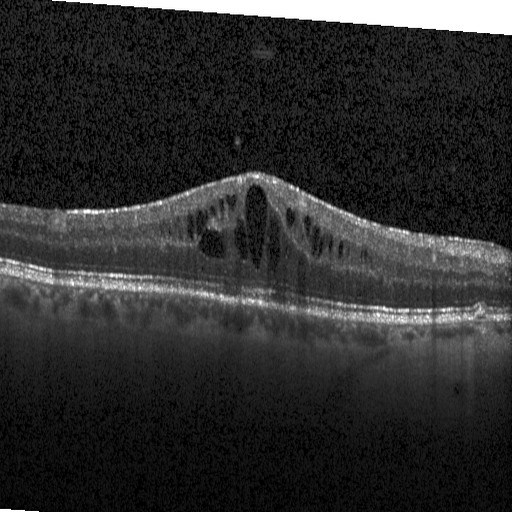 SD-OCT. Through the macula. Optical coherence tomography scan. This B-scan demonstrates DME.